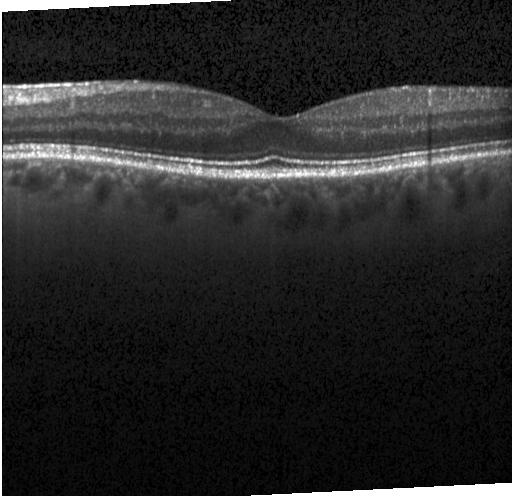

Impression: no CNV, no DME, and no drusen.